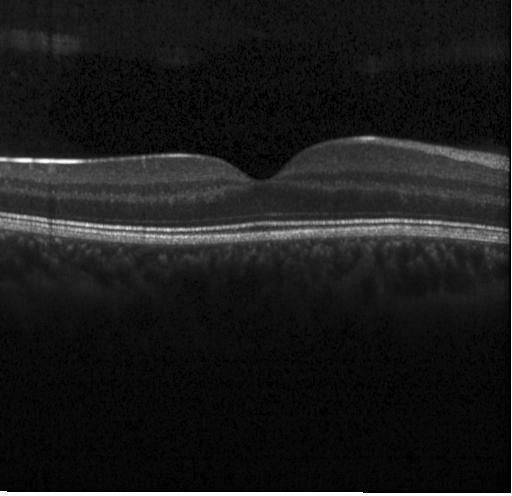 Spectral-domain OCT B-scan: no choroidal neovascularization, diabetic macular edema, or drusen.